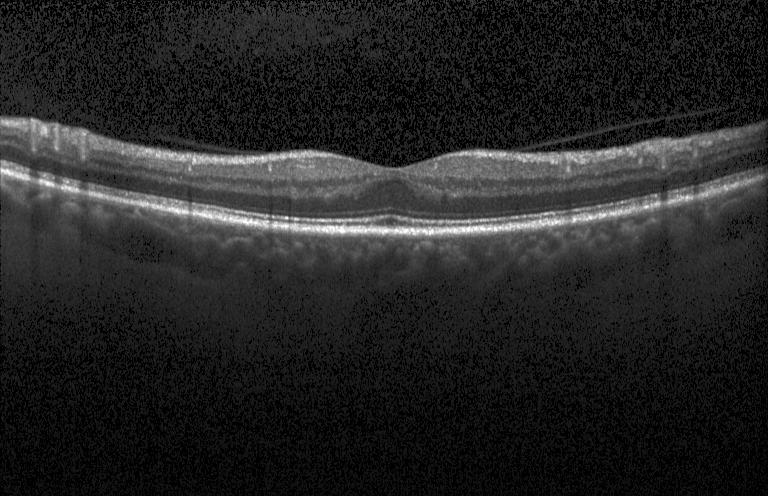

Retinal OCT cross-section, instrument: Heidelberg Spectralis, fovea-centered. Diagnosis: no choroidal neovascularization, no diabetic macular edema, and no drusen.